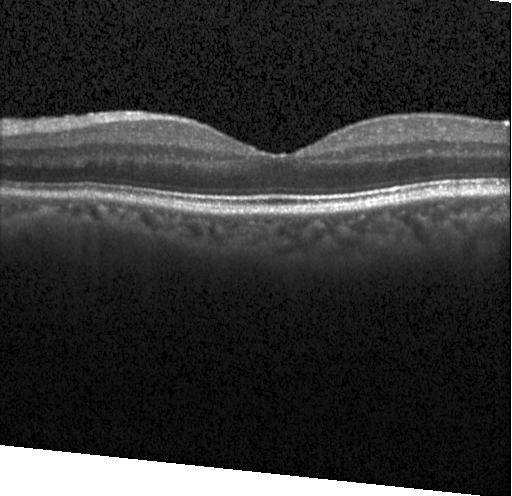 Finding: no choroidal neovascularization, no diabetic macular edema, and no drusen.